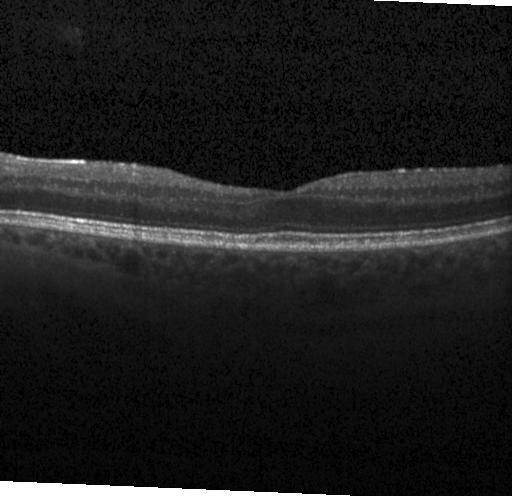
OCT finding: neither choroidal neovascularization, diabetic macular edema, nor drusen.